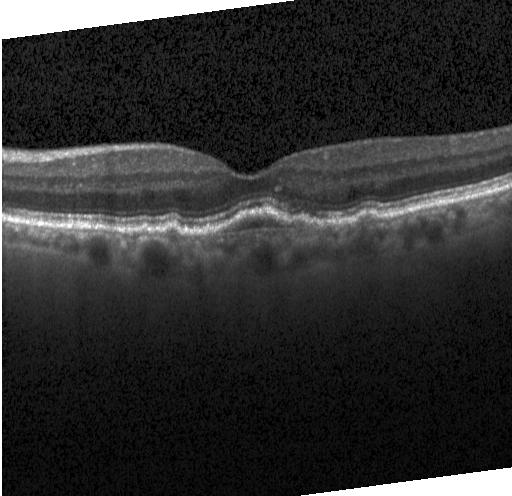
Macular scan. Retinal OCT cross-section.
Diagnosis: CNV.